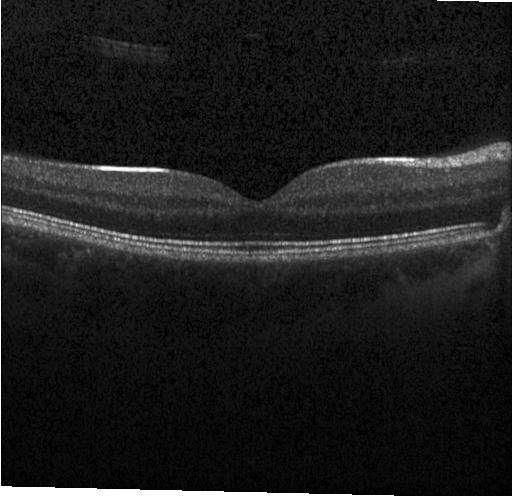

OCT B-scan — Finding: no evidence of choroidal neovascularization, diabetic macular edema, or drusen.